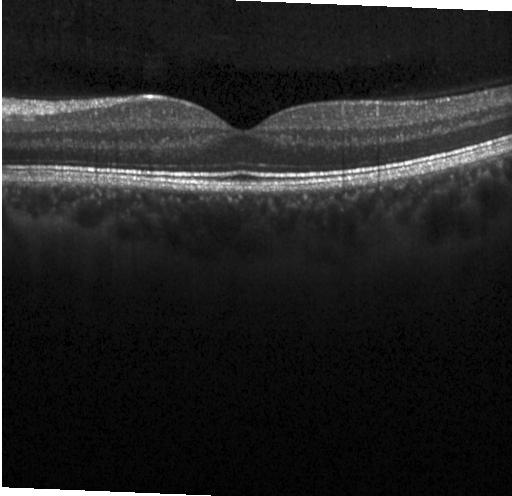
Optical coherence tomography scan — Finding: no choroidal neovascularization, no diabetic macular edema, and no drusen.